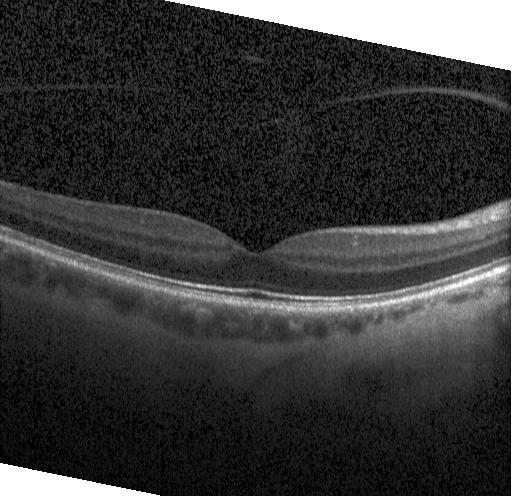 Centered on the fovea. OCT line scan
Dx: no evidence of CNV, DME, or drusen.